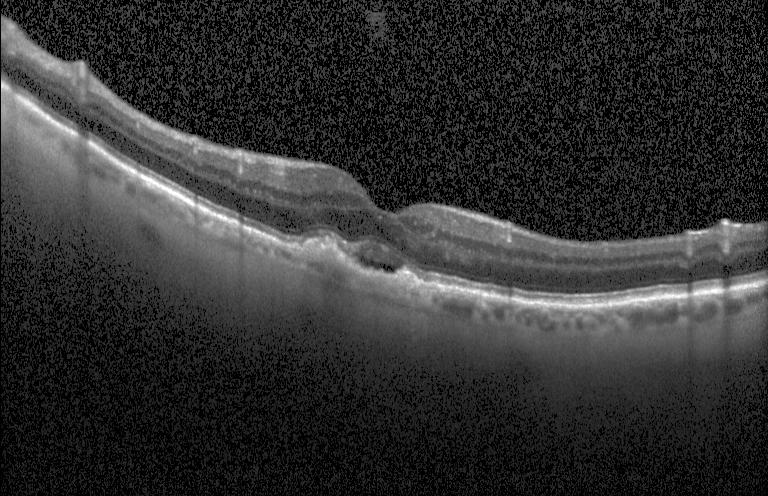 Heidelberg Spectralis. Retinal OCT B-scan. SD-OCT.
Finding: a choroidal neovascular membrane.